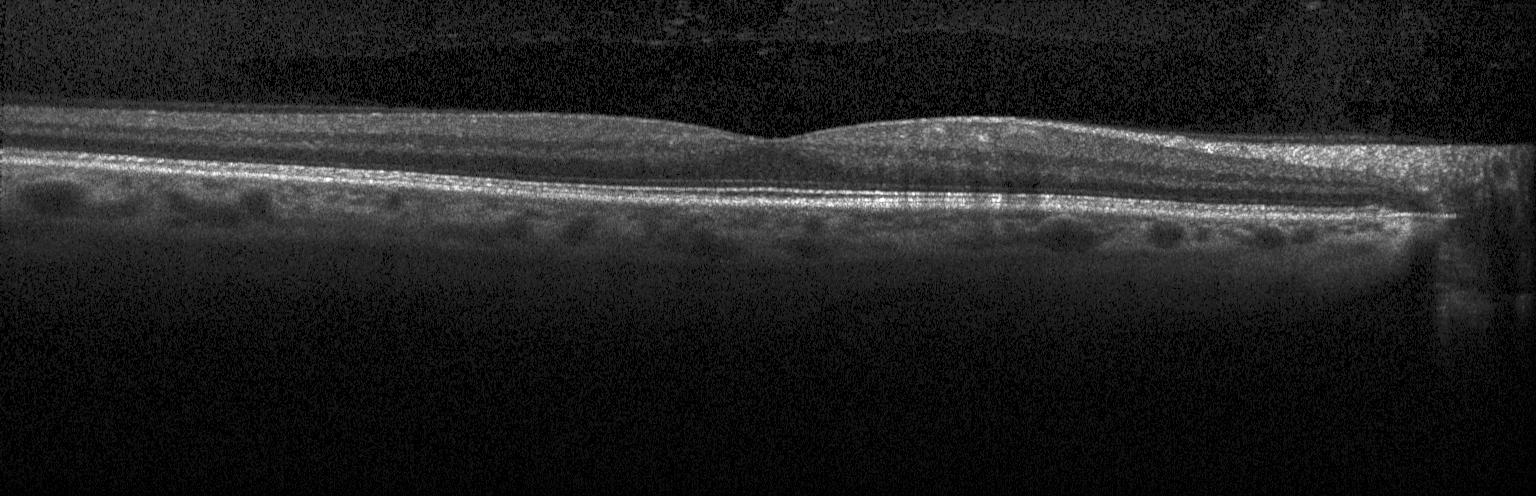

Optical coherence tomography B-scan
Diagnosis: no choroidal neovascularization, no diabetic macular edema, and no drusen.